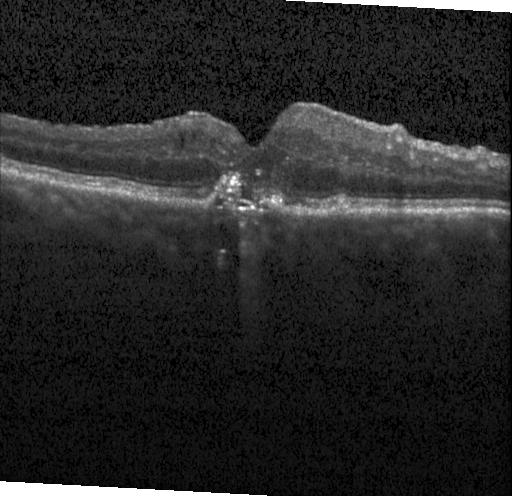
Macular OCT: a choroidal neovascular membrane.